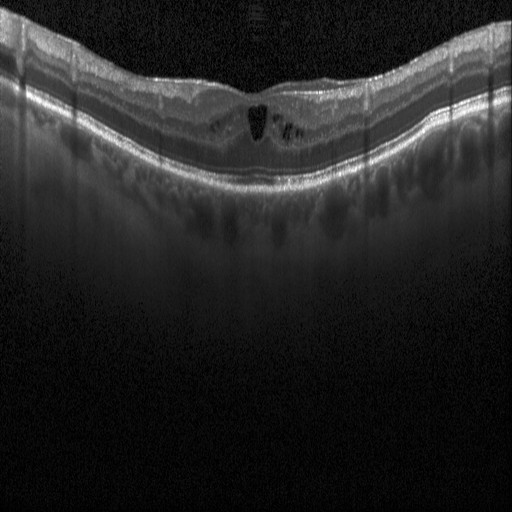

Diagnosis: diabetic macular edema.